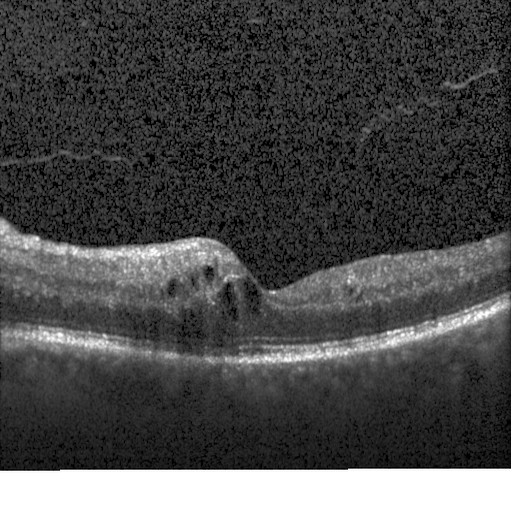 Macular OCT: DME.